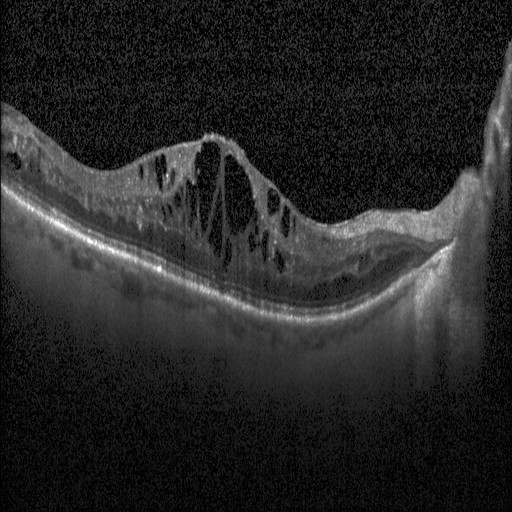
Optical coherence tomography B-scan.
Macular OCT: diabetic macular edema.